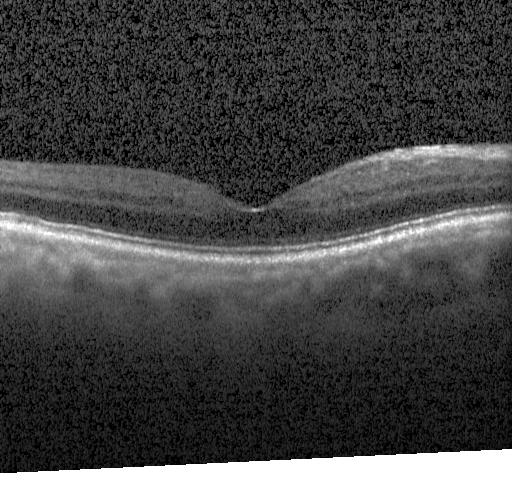
Retinal OCT B-scan
Dx: no evidence of choroidal neovascularization, diabetic macular edema, or drusen.